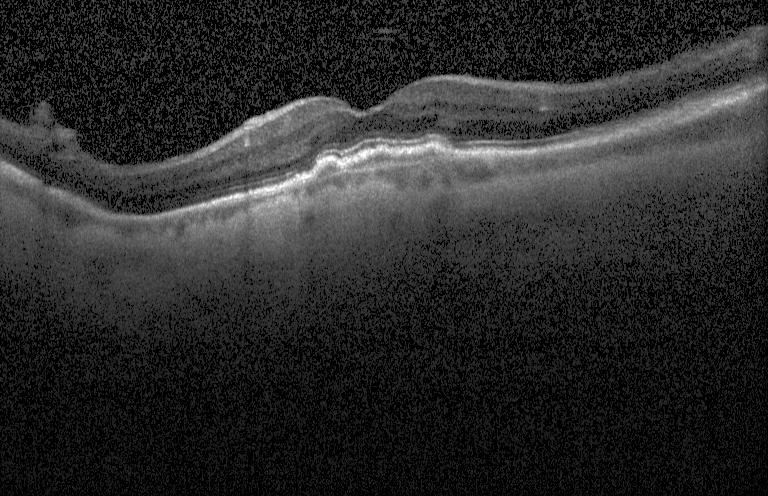

Heidelberg Spectralis OCT system, retinal OCT cross-section. OCT finding: choroidal neovascularization (CNV).